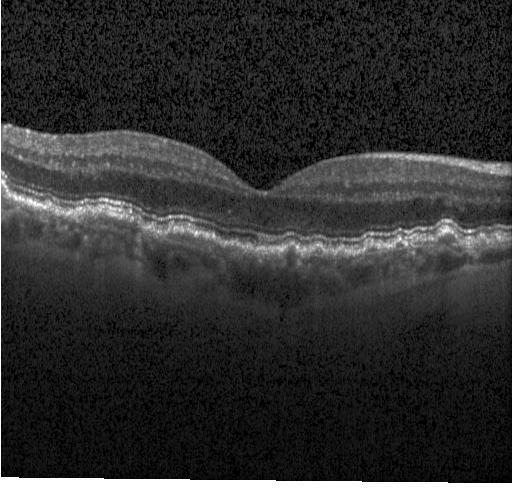 Centered on the fovea. OCT line scan. Diagnosis: sub-RPE drusenoid deposits.